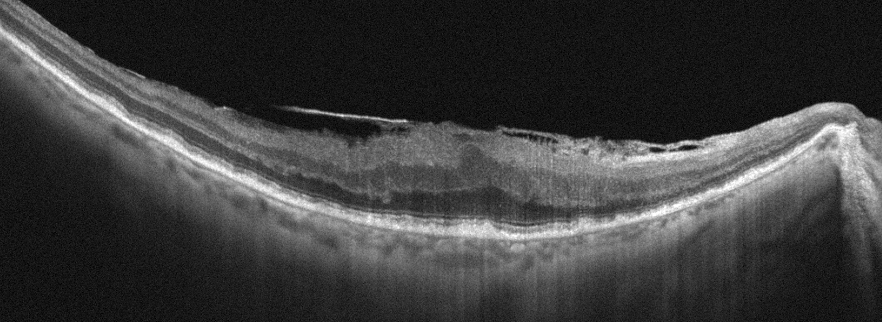
Retinal OCT B-scan. Macular scan. The scan shows epiretinal membrane.